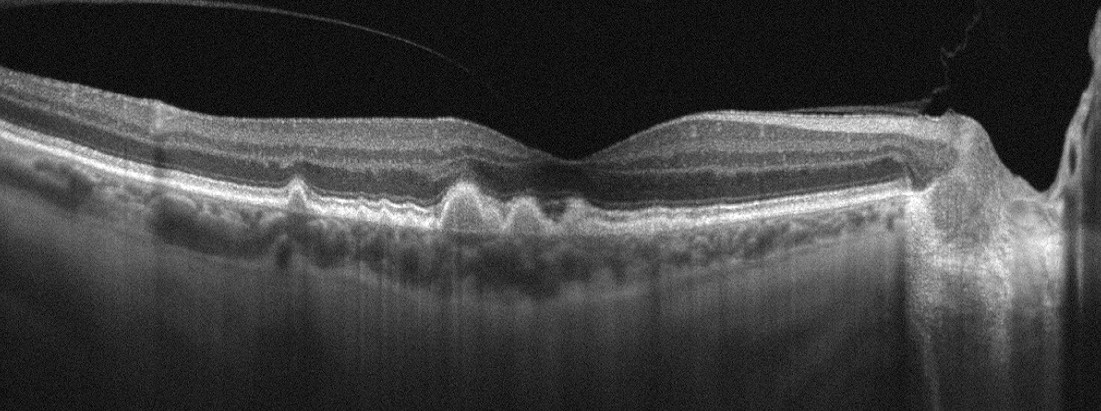
Optovue Avanti RTVue XR · OCT line scan · fovea-centered
The scan shows AMD.